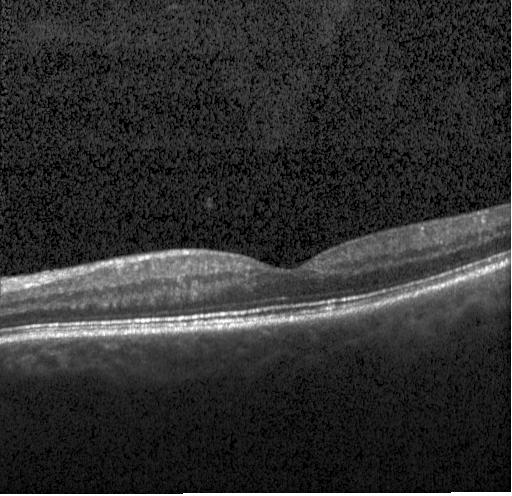 Impression: neither CNV, DME, nor drusen.